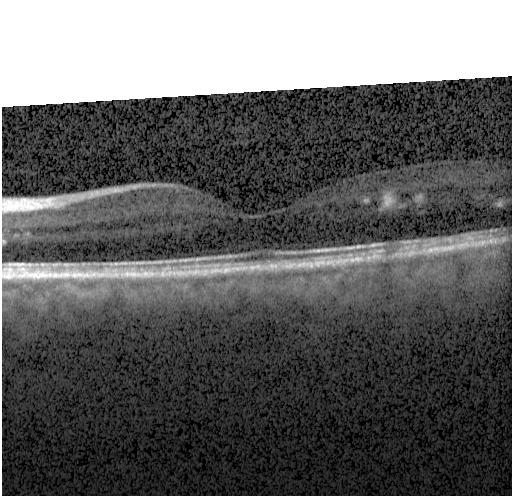

Finding: no CNV, DME, or drusen.